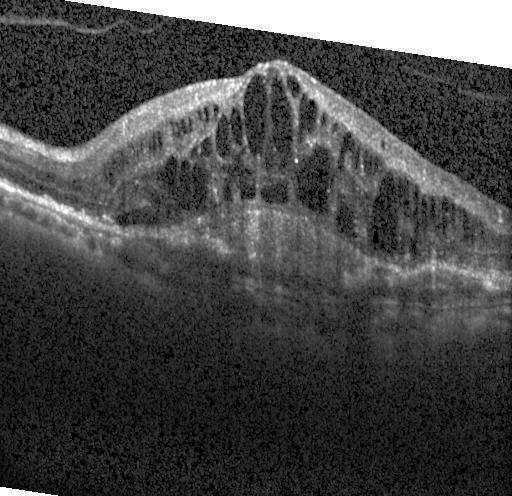 Spectral-domain optical coherence tomography; optical coherence tomography scan; Heidelberg Spectralis; horizontal scan through the fovea. Dx: CNV.